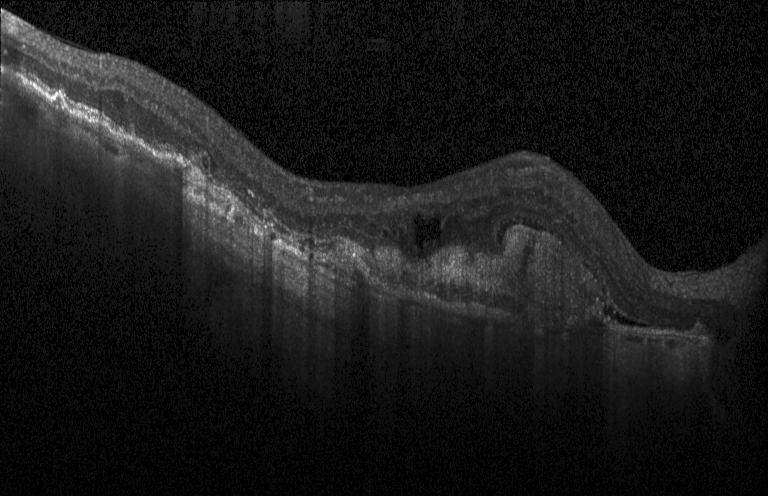
Optical coherence tomography B-scan — OCT finding: choroidal neovascularization.